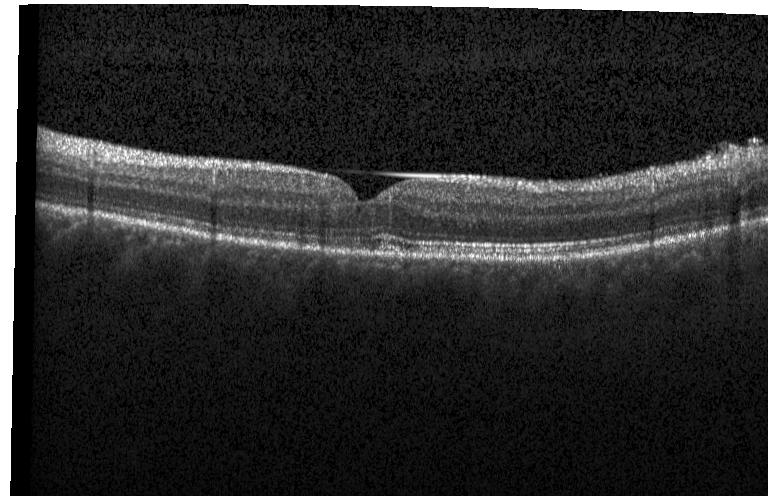
Retinal OCT B-scan · spectral-domain optical coherence tomography · through the macula · Heidelberg Spectralis OCT system. OCT finding: no CNV, no DME, and no drusen.